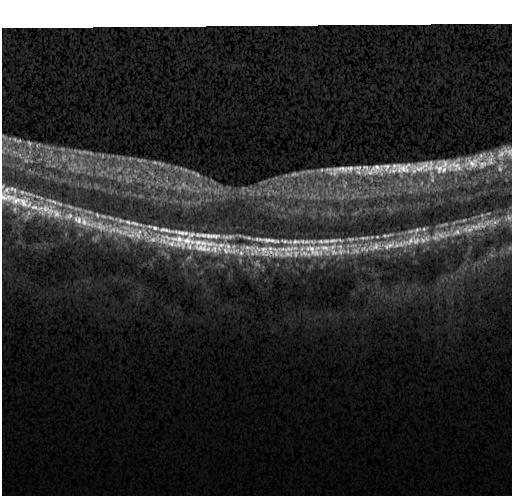 Finding: no choroidal neovascularization, diabetic macular edema, or drusen.